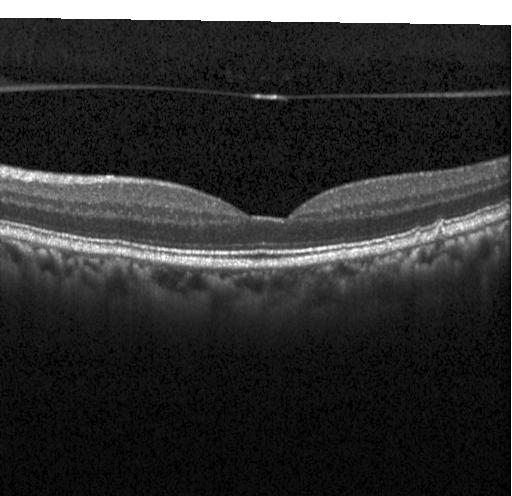 OCT line scan · SD-OCT — Assessment: drusen.